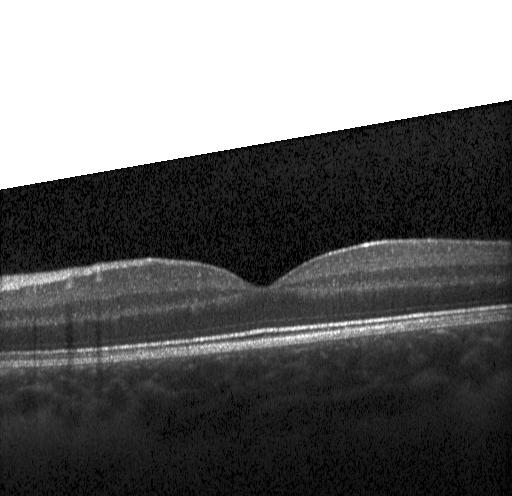 The scan shows neither choroidal neovascularization, diabetic macular edema, nor drusen.